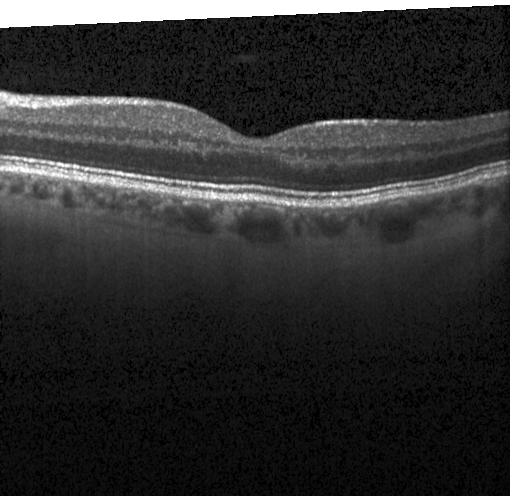

OCT B-scan · spectral-domain optical coherence tomography · Heidelberg Spectralis
No CNV, DME, or drusen.